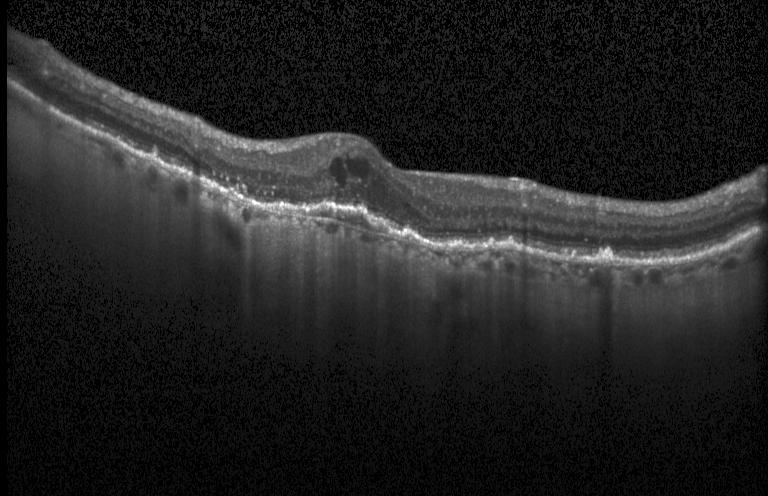
Retinal OCT B-scan.
Finding: choroidal neovascularization (CNV).